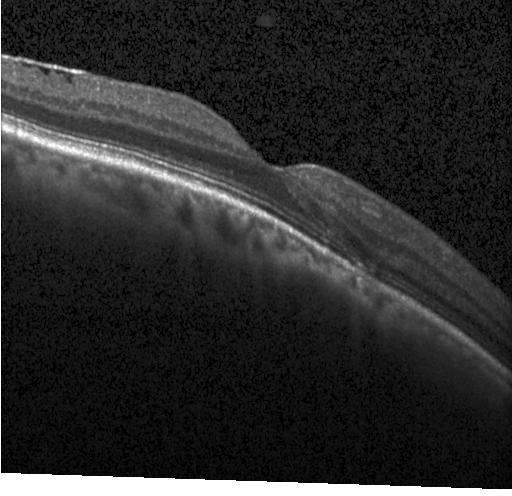

Optical coherence tomography scan.
OCT finding: no choroidal neovascularization, no diabetic macular edema, and no drusen.